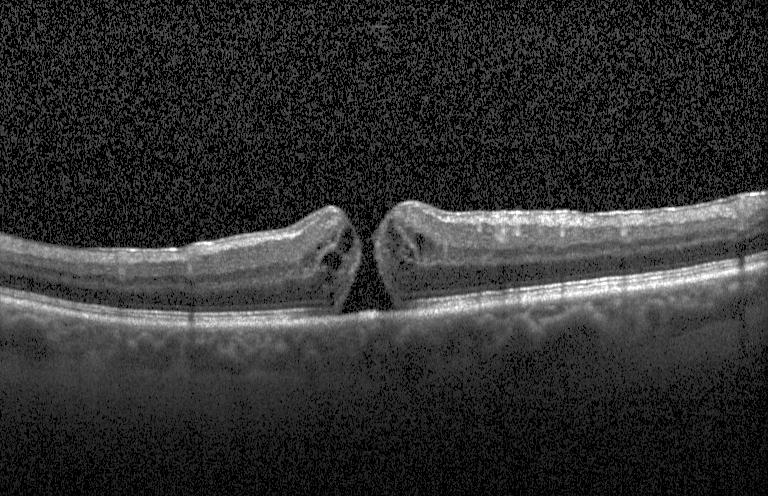 Assessment: diabetic macular edema (DME).